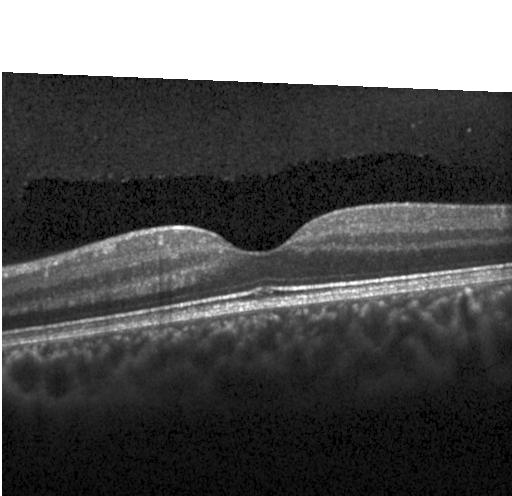

Optical coherence tomography scan; through the macula.
The scan shows no evidence of choroidal neovascularization, diabetic macular edema, or drusen.